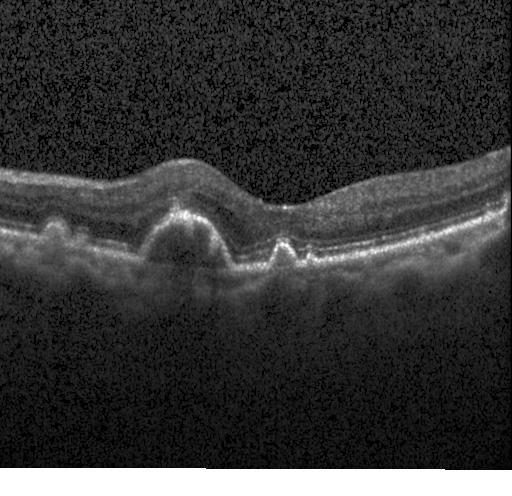

Impression: drusen.